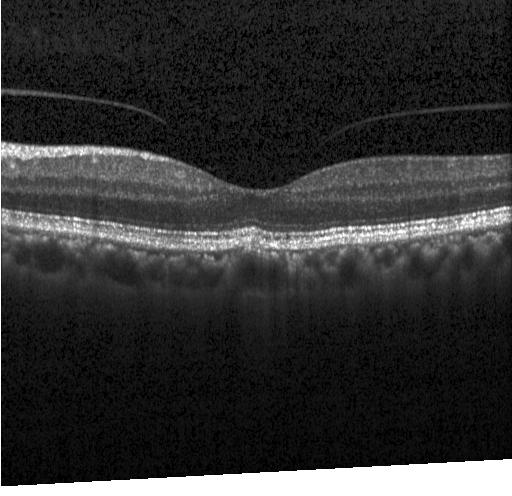 Optical coherence tomography B-scan, horizontal scan through the fovea
Assessment: no CNV, no DME, and no drusen.